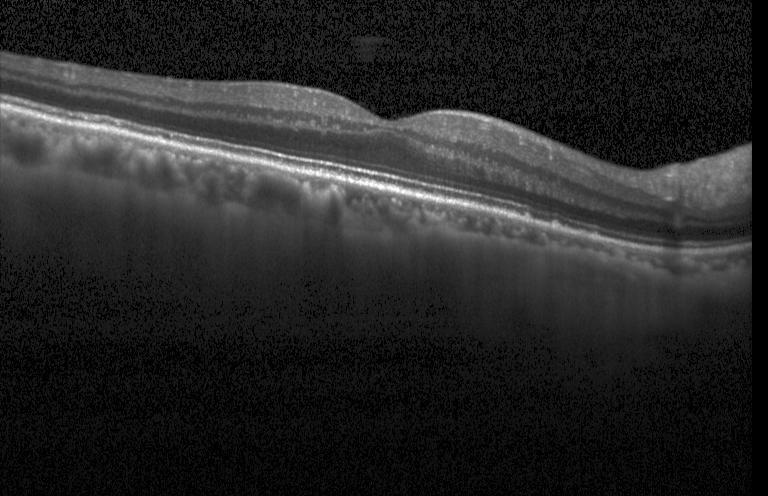
Diagnosis: no choroidal neovascularization, no diabetic macular edema, and no drusen.